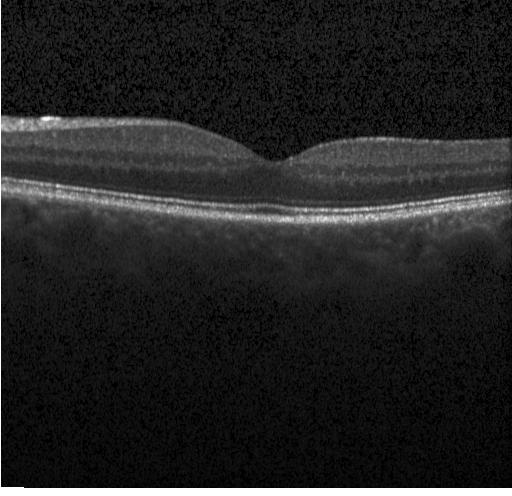

Macular scan · acquired on a Heidelberg Spectralis · SD-OCT · OCT B-scan.
Assessment: no evidence of choroidal neovascularization, diabetic macular edema, or drusen.